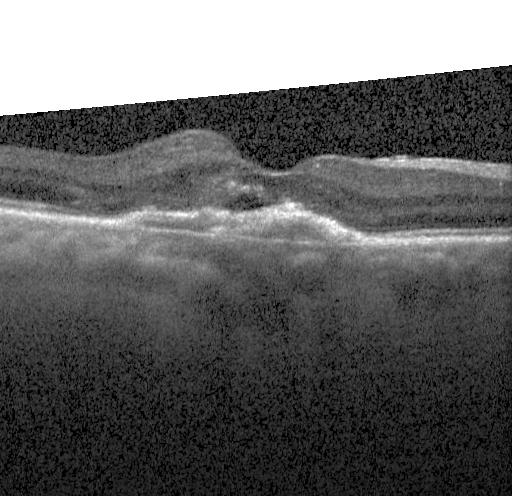
OCT B-scan — OCT finding: choroidal neovascularization.